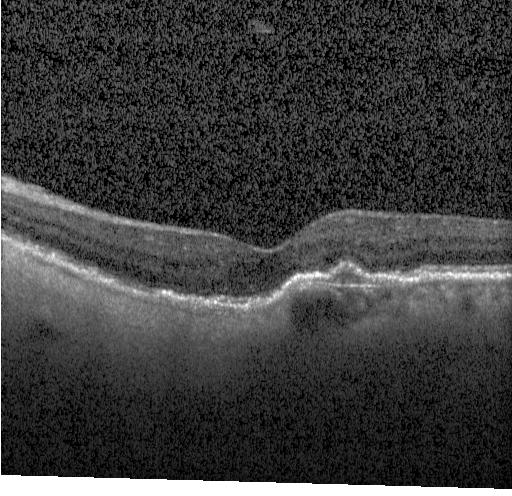 Finding: a choroidal neovascular membrane.